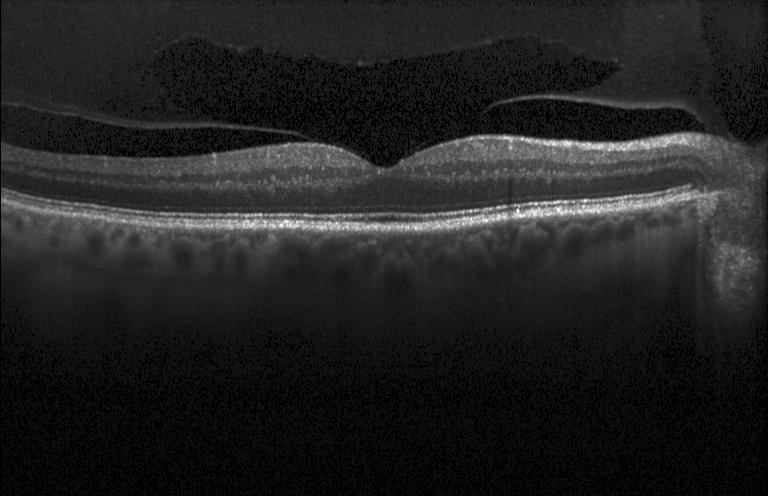 Retinal OCT cross-section · fovea-centered. Macular OCT: no evidence of choroidal neovascularization, diabetic macular edema, or drusen.